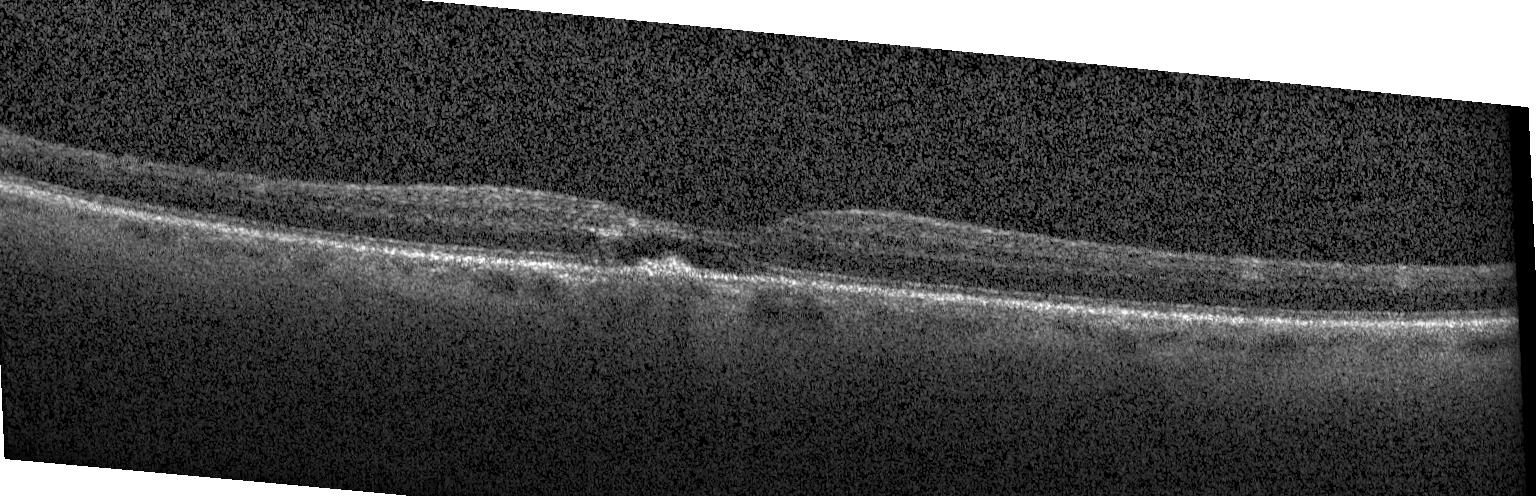
Optical coherence tomography B-scan. SD-OCT. Horizontal scan through the fovea.
Dx: a choroidal neovascular membrane.